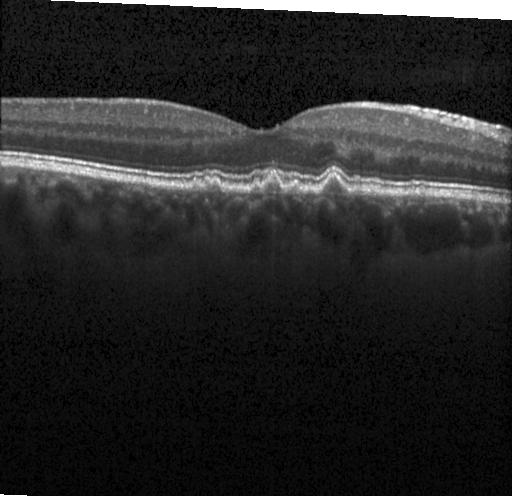

OCT B-scan showing multiple drusen.